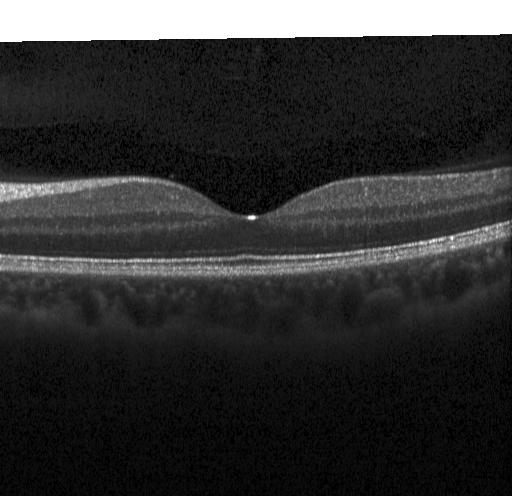

Through the macula; OCT line scan; spectral-domain optical coherence tomography — Assessment: neither choroidal neovascularization, diabetic macular edema, nor drusen.